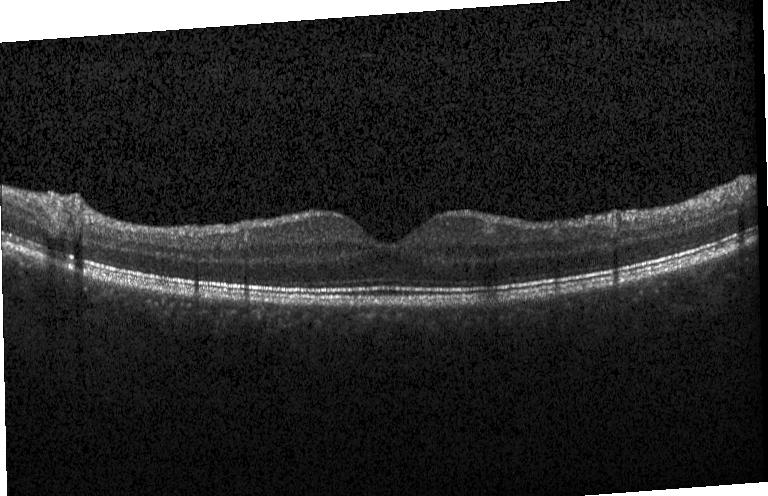

Through the macula. Retinal OCT B-scan. Heidelberg Spectralis. Spectral-domain optical coherence tomography
Diagnosis: no CNV, no DME, and no drusen.